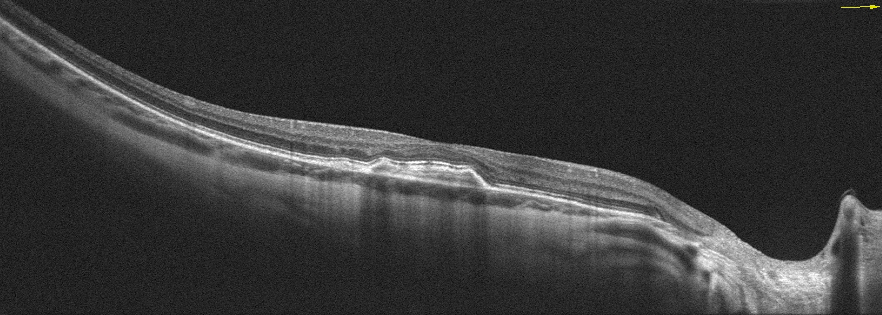

Instrument: Optovue Avanti RTVue XR; OCT line scan.
Assessment: age-related macular degeneration.